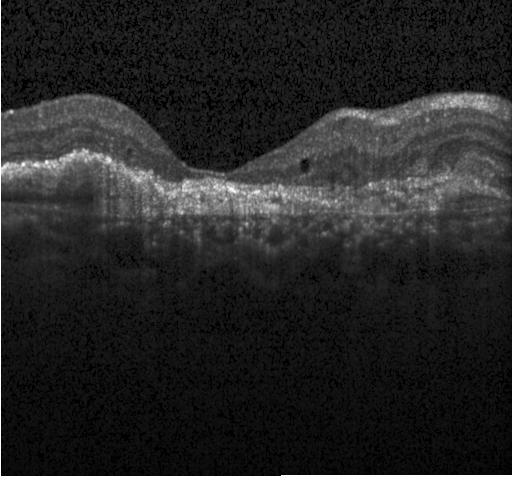 Retinal OCT B-scan. Macular scan. Acquired on a Heidelberg Spectralis. Spectral-domain OCT — Finding: a choroidal neovascular membrane.